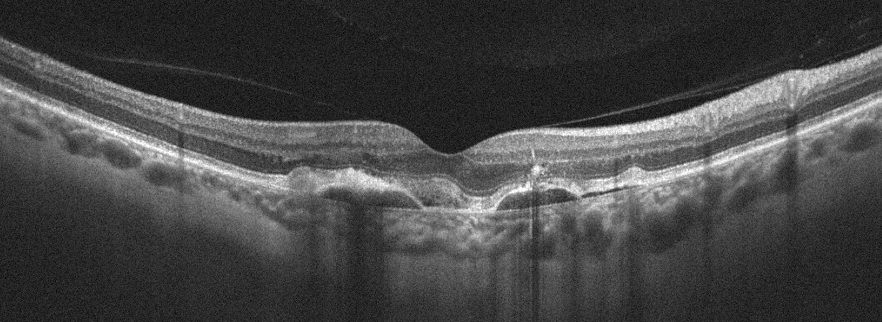
OD, acquired on an Optovue Avanti RTVue XR, macular scan, optical coherence tomography B-scan.
Impression: age-related macular degeneration.